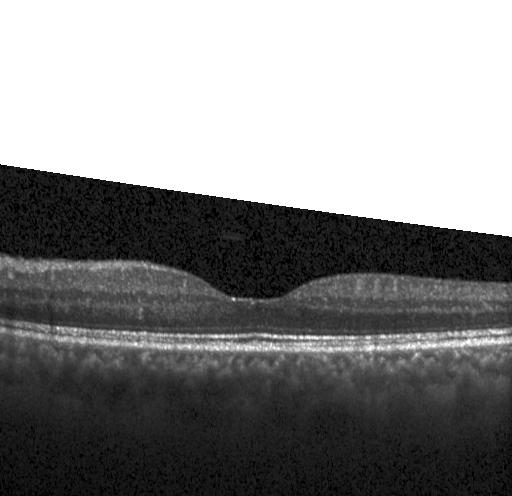 Heidelberg Spectralis · macular scan · retinal OCT cross-section · SD-OCT.
Neither choroidal neovascularization, diabetic macular edema, nor drusen.